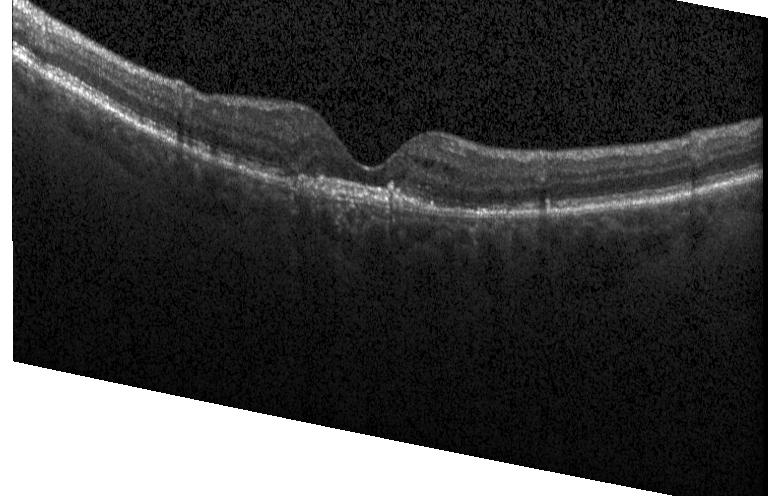
Instrument: Heidelberg Spectralis; optical coherence tomography B-scan; macular scan.
A choroidal neovascular membrane.